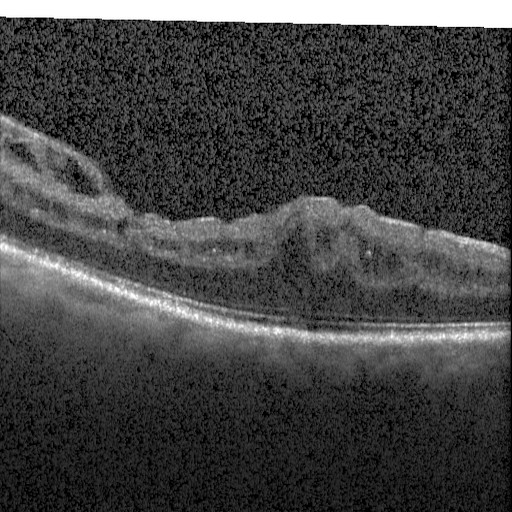 Retinal OCT B-scan; instrument: Heidelberg Spectralis. Impression: DME.